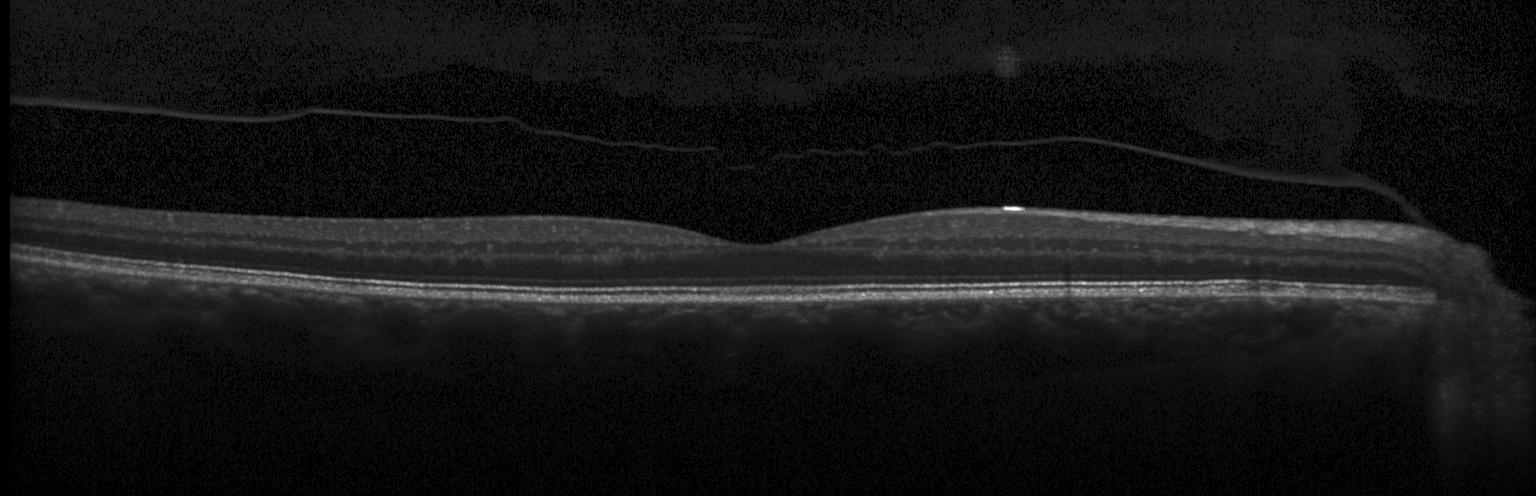 Heidelberg Spectralis OCT system; OCT line scan; SD-OCT; fovea-centered.
No evidence of choroidal neovascularization, diabetic macular edema, or drusen.